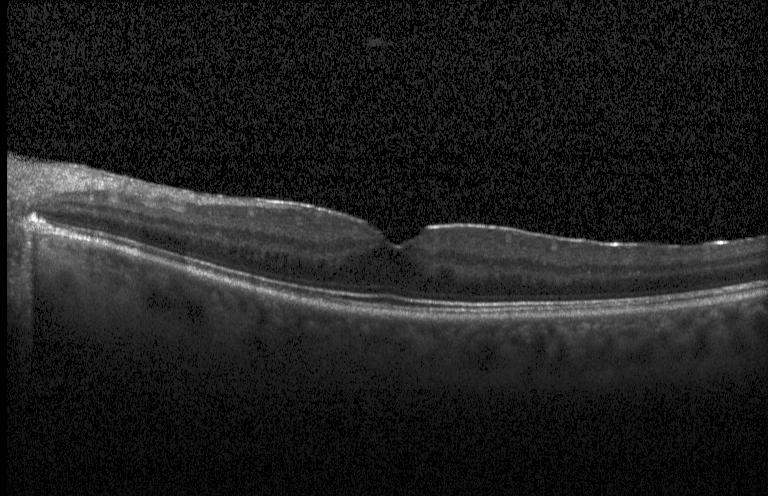
Impression: no evidence of CNV, DME, or drusen.